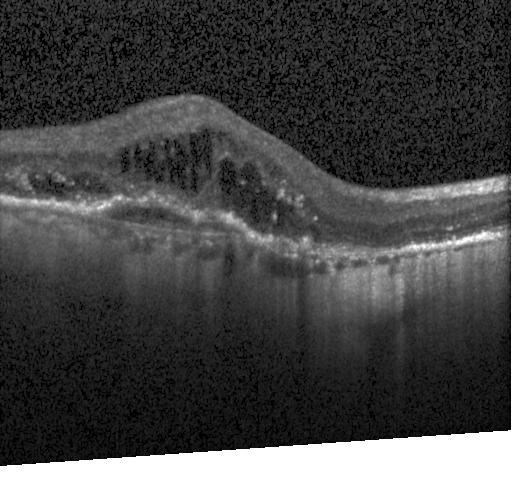
Optical coherence tomography B-scan. Dx: a choroidal neovascular membrane.